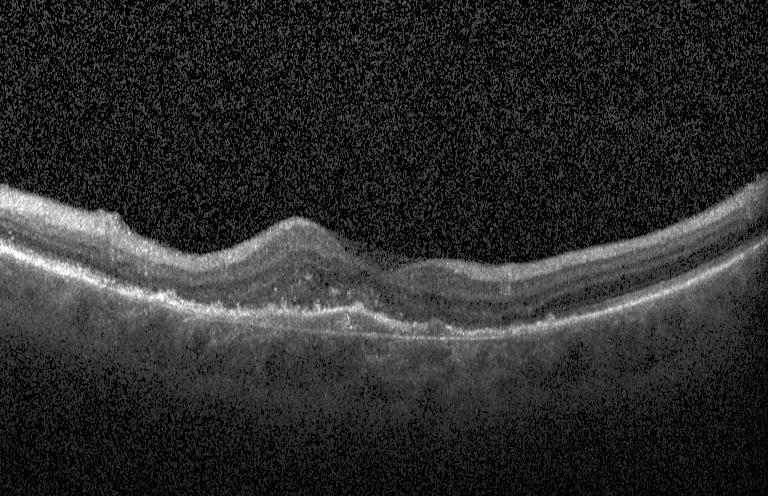 Through the macula; Heidelberg Spectralis OCT system; optical coherence tomography B-scan
Assessment: choroidal neovascularization (CNV).